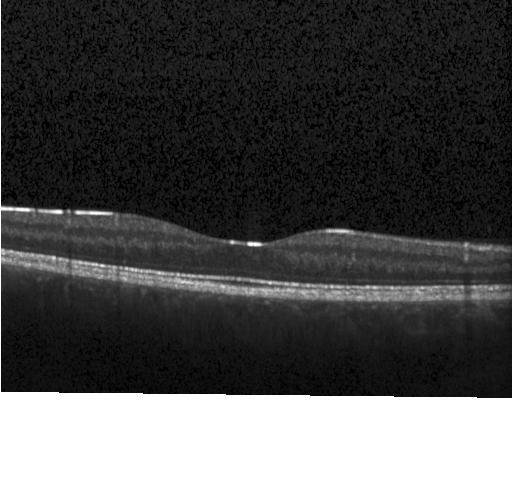
OCT B-scan. Dx: no choroidal neovascularization, diabetic macular edema, or drusen.